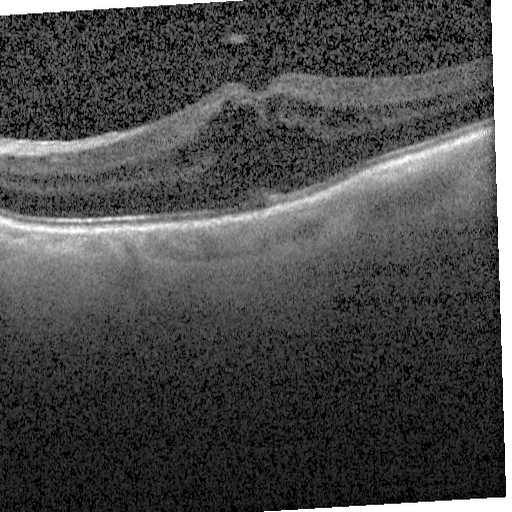

The scan shows DME.